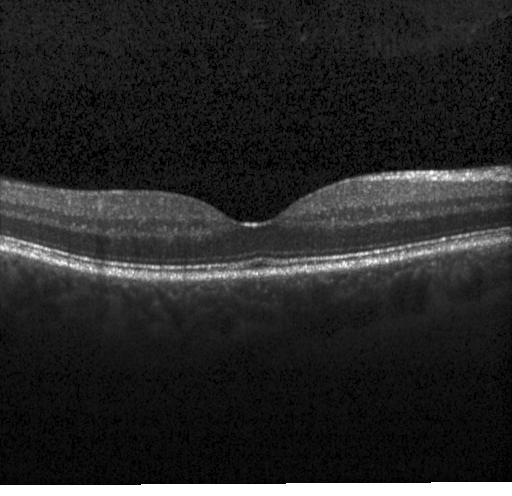

Retinal OCT cross-section · spectral-domain OCT · through the macula
Impression: no choroidal neovascularization, no diabetic macular edema, and no drusen.